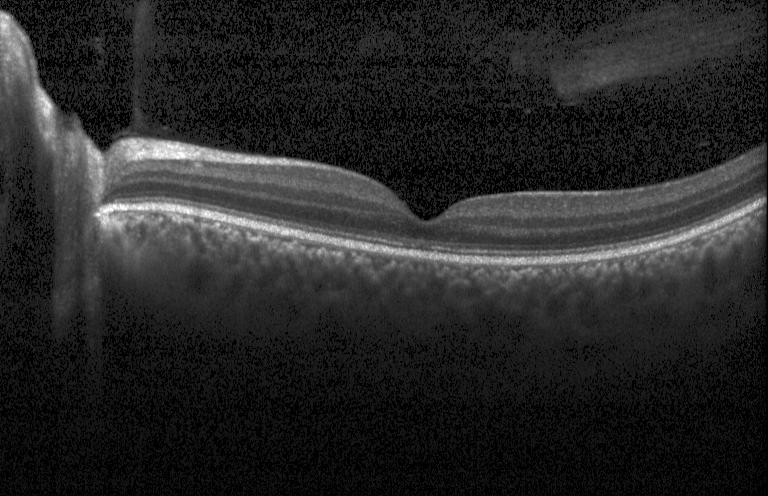

OCT B-scan showing no evidence of choroidal neovascularization, diabetic macular edema, or drusen.